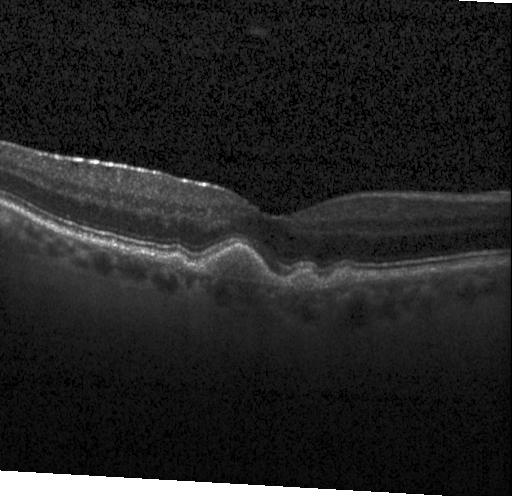 Sub-RPE drusenoid deposits.